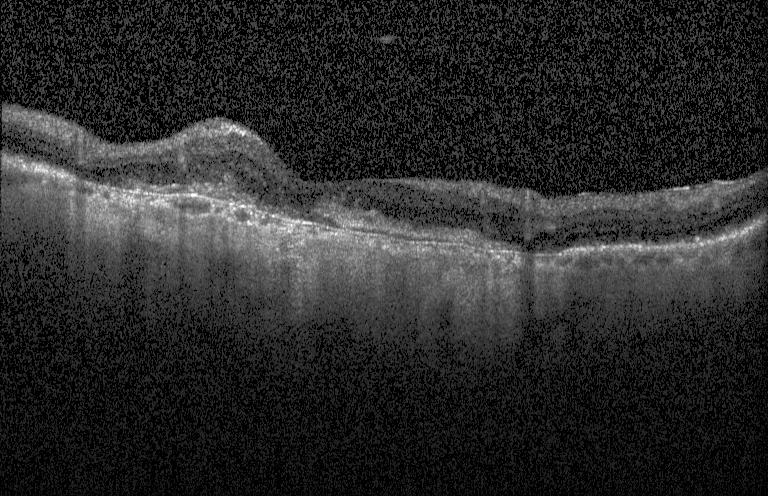

The scan shows a choroidal neovascular membrane.